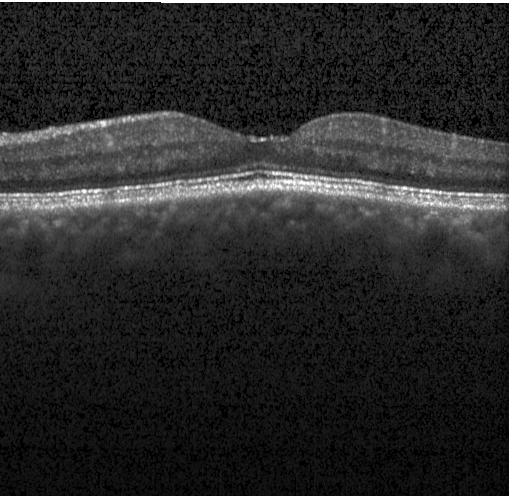

Horizontal scan through the fovea; spectral-domain optical coherence tomography; Heidelberg Spectralis OCT system; retinal OCT B-scan — No CNV, DME, or drusen.